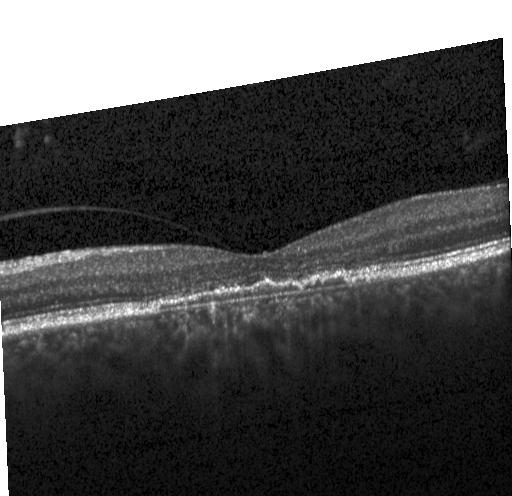

Diagnosis: CNV.